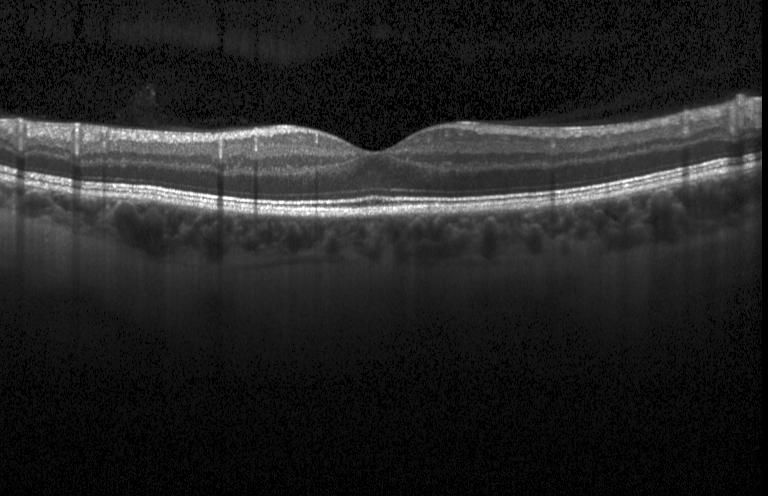
OCT finding: no CNV, DME, or drusen.